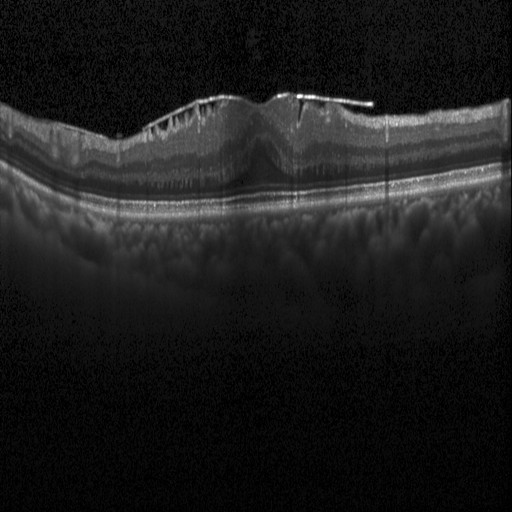 Spectral-domain OCT · horizontal scan through the fovea · retinal OCT cross-section · Heidelberg Spectralis OCT system — The scan shows diabetic macular edema.